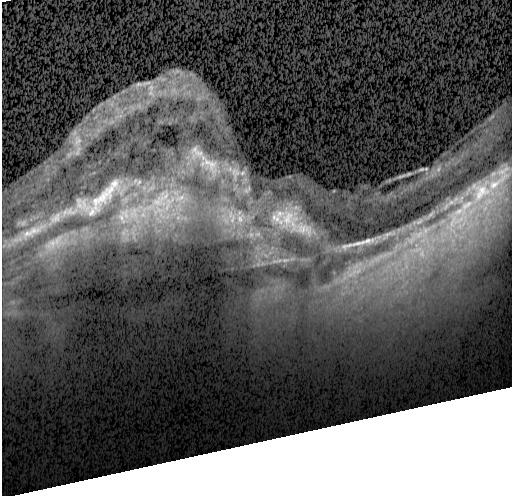 OCT B-scan — OCT finding: a choroidal neovascular membrane.